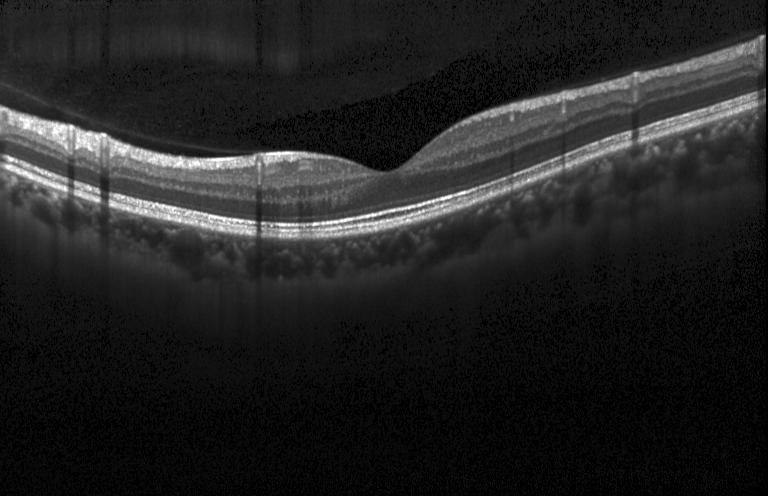 OCT B-scan. Diagnosis: no evidence of choroidal neovascularization, diabetic macular edema, or drusen.